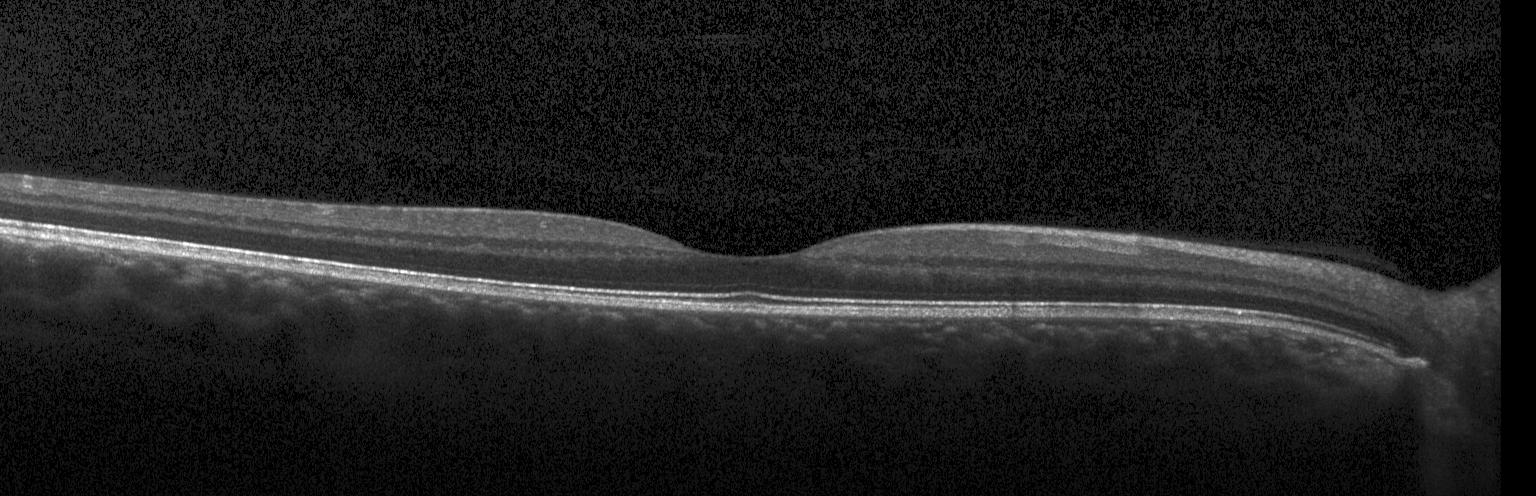

Spectral-domain optical coherence tomography, fovea-centered, retinal OCT cross-section — This B-scan demonstrates no choroidal neovascularization, diabetic macular edema, or drusen.